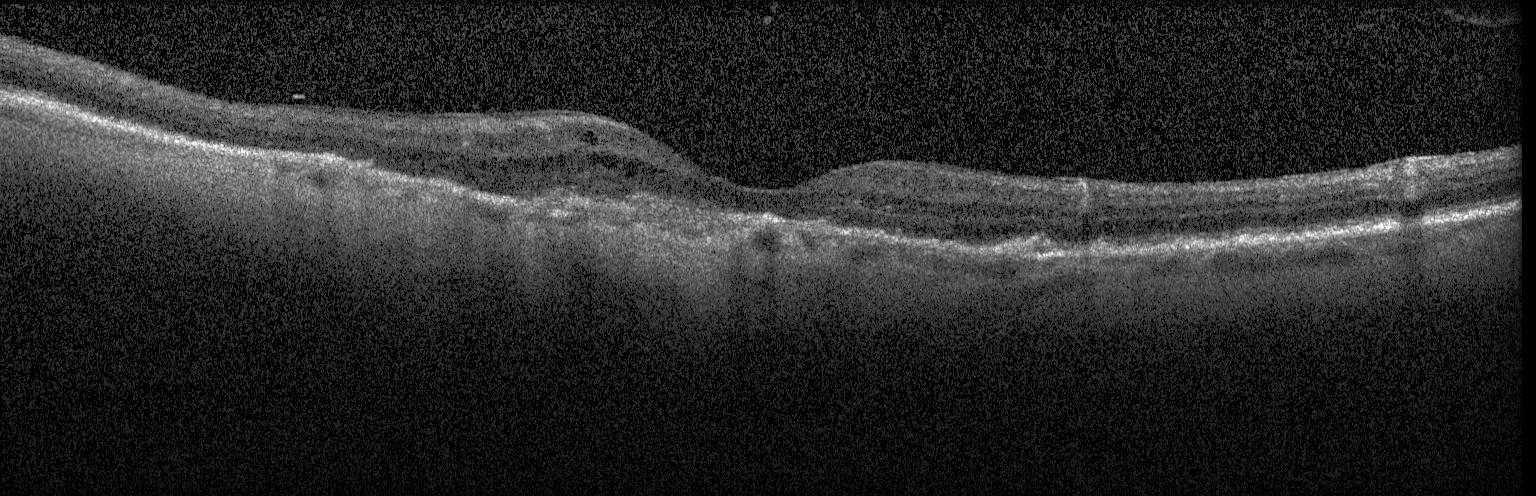
OCT scan showing CNV.